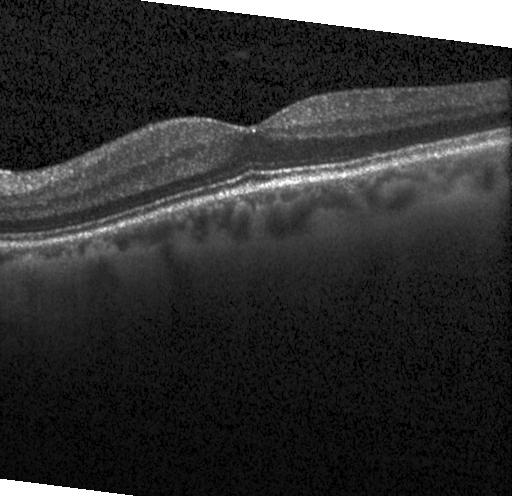

OCT scan showing no evidence of CNV, DME, or drusen.